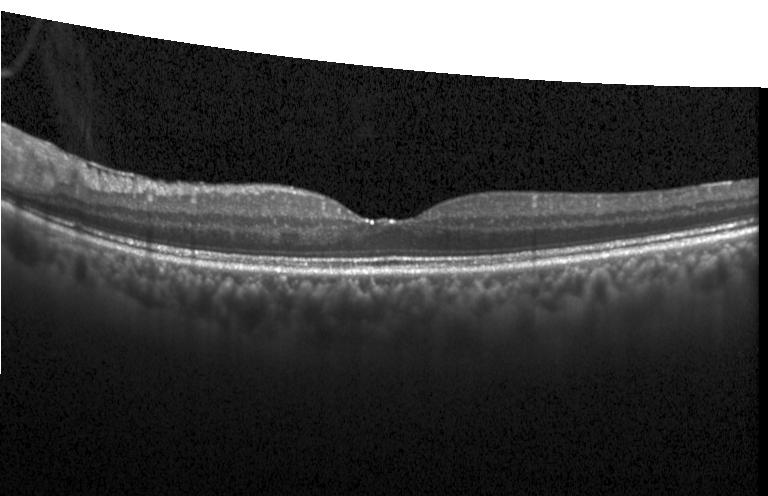
Spectral-domain OCT; acquired on a Heidelberg Spectralis; optical coherence tomography B-scan; horizontal scan through the fovea — No choroidal neovascularization, diabetic macular edema, or drusen.